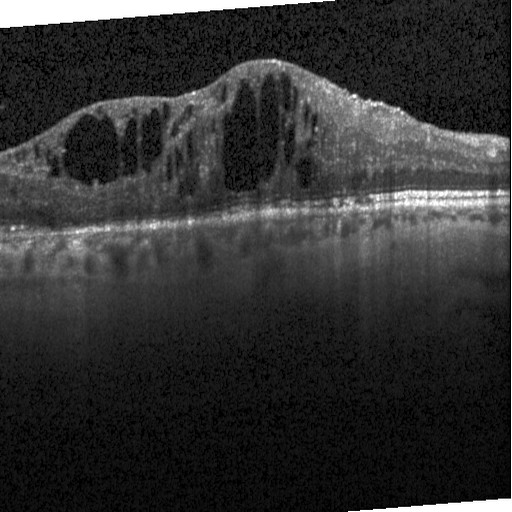 Impression: diabetic macular edema.